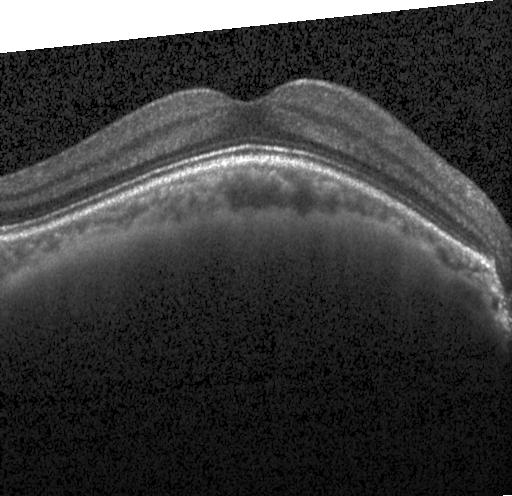 OCT line scan, through the macula
No evidence of choroidal neovascularization, diabetic macular edema, or drusen.